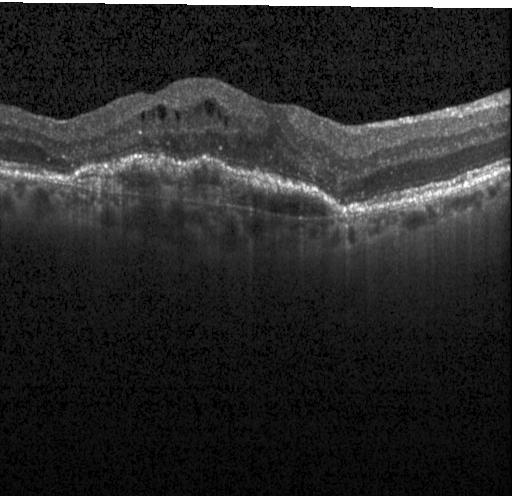

OCT finding: CNV.